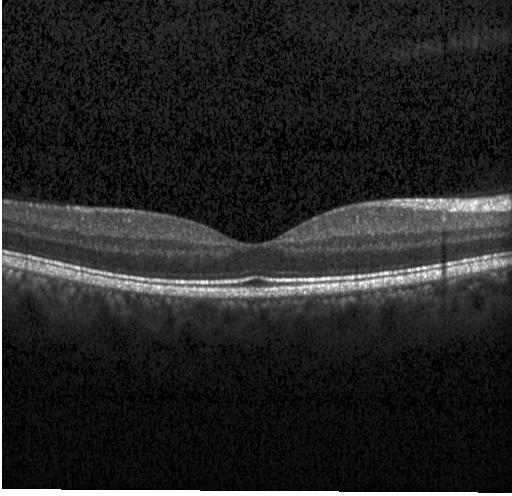
Centered on the fovea; optical coherence tomography B-scan.
Diagnosis: no choroidal neovascularization, no diabetic macular edema, and no drusen.